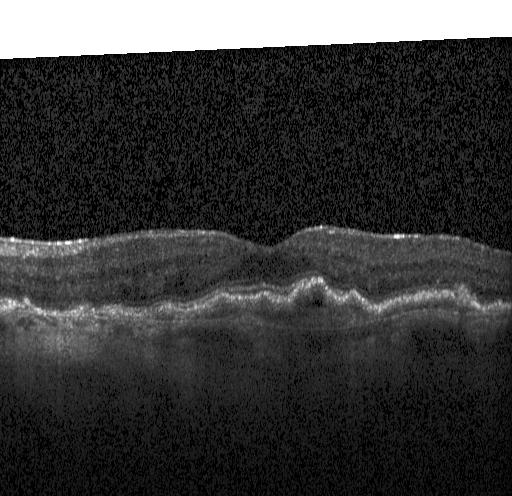

A choroidal neovascular membrane.